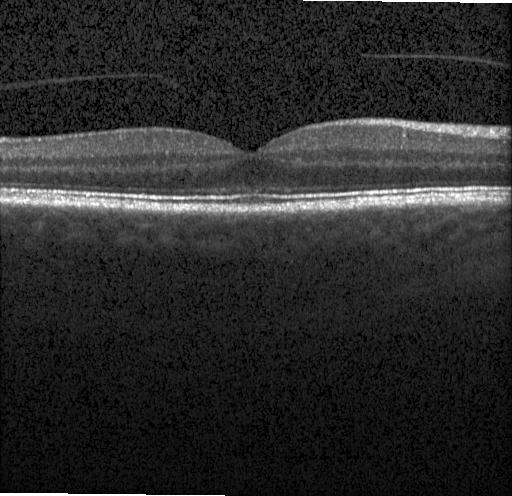

OCT B-scan showing neither choroidal neovascularization, diabetic macular edema, nor drusen.